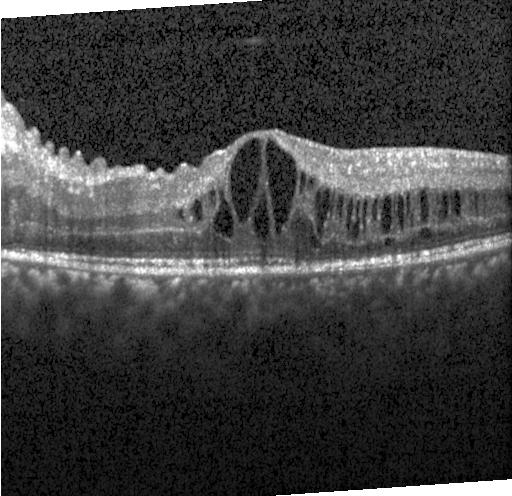

Finding: diabetic macular edema.